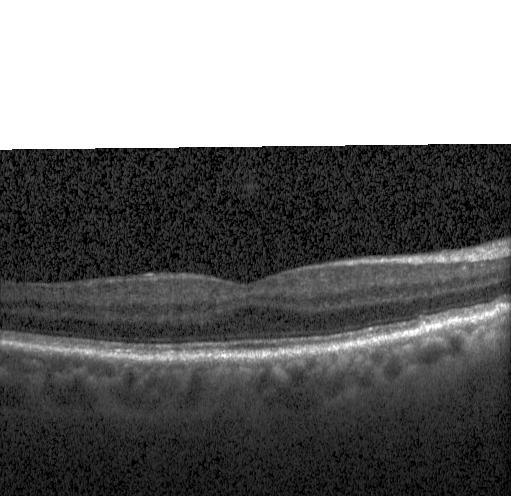

Optical coherence tomography scan — Finding: neither CNV, DME, nor drusen.